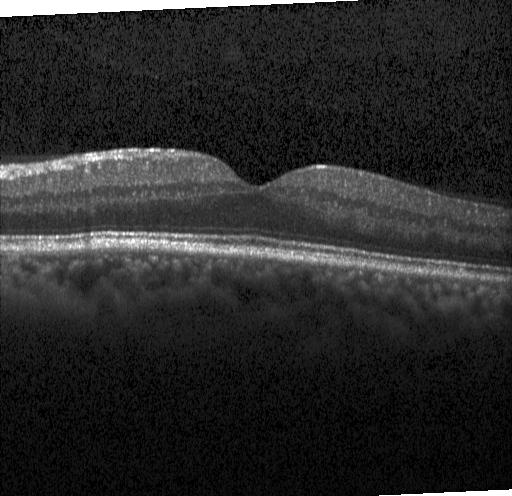
Centered on the fovea, optical coherence tomography B-scan, SD-OCT, Heidelberg Spectralis — The scan shows no choroidal neovascularization, diabetic macular edema, or drusen.